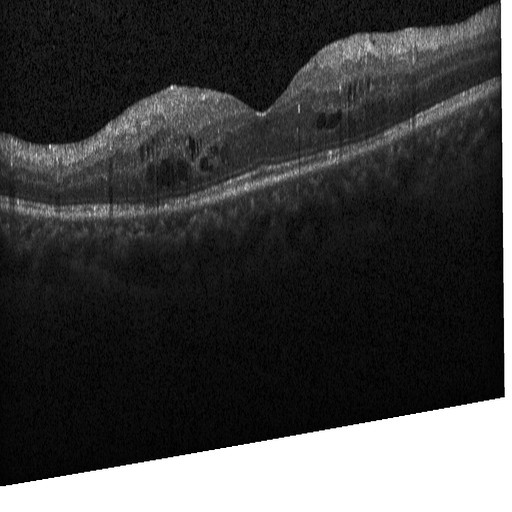

Retinal OCT cross-section showing diabetic macular edema (DME).